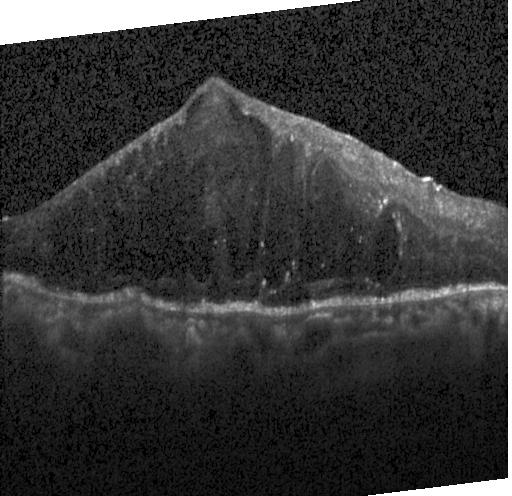 Instrument: Heidelberg Spectralis · optical coherence tomography scan. The scan shows diabetic macular edema.